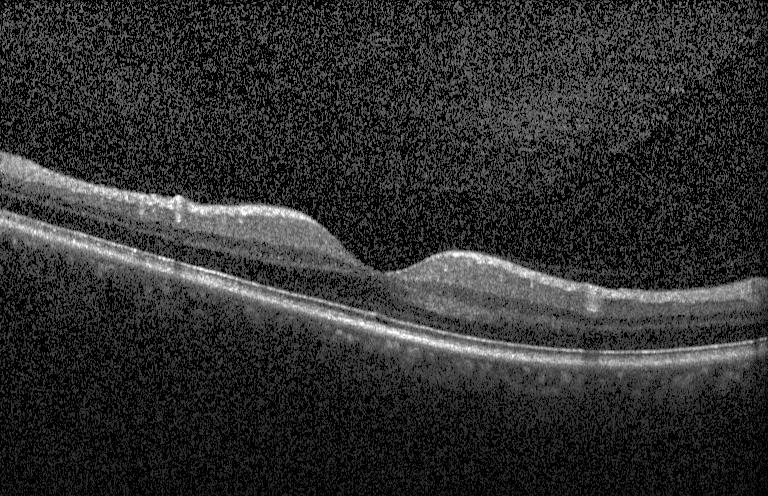

Dx: no choroidal neovascularization, diabetic macular edema, or drusen.